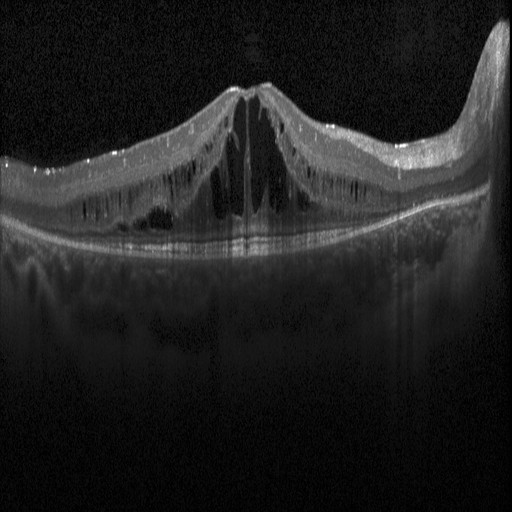
Spectral-domain OCT B-scan: diabetic macular edema.